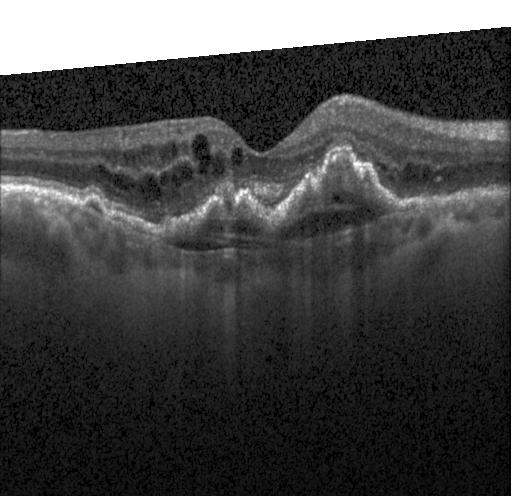

Through the macula, optical coherence tomography B-scan — Dx: choroidal neovascularization.